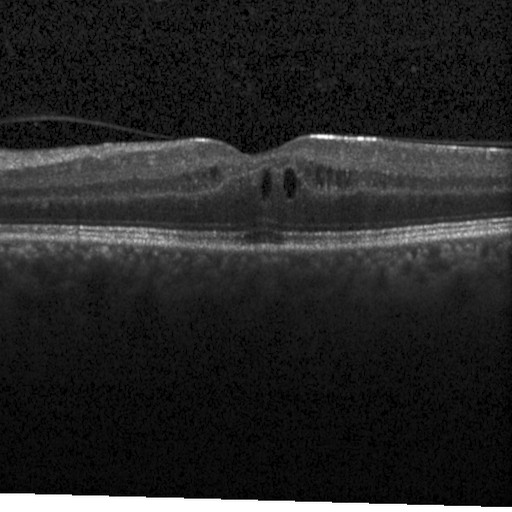

Retinal OCT cross-section; SD-OCT.
Assessment: DME.